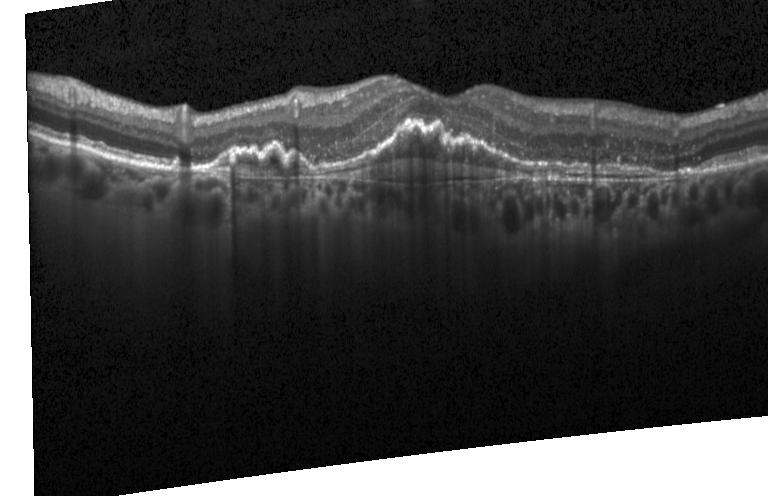 Spectral-domain OCT · retinal OCT cross-section · macular scan · Heidelberg Spectralis — Macular OCT: a choroidal neovascular membrane.